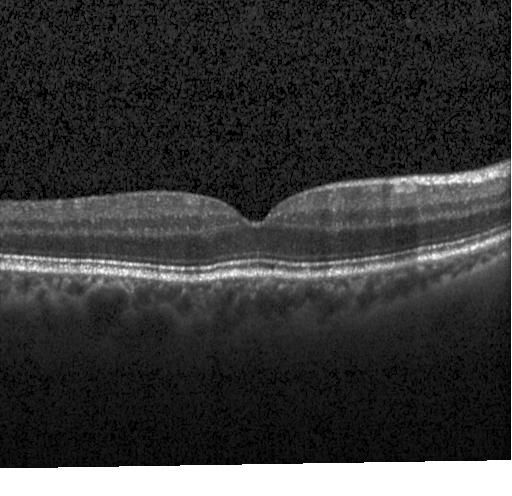

Instrument: Heidelberg Spectralis; spectral-domain optical coherence tomography; macular scan; OCT B-scan — OCT finding: no choroidal neovascularization, diabetic macular edema, or drusen.